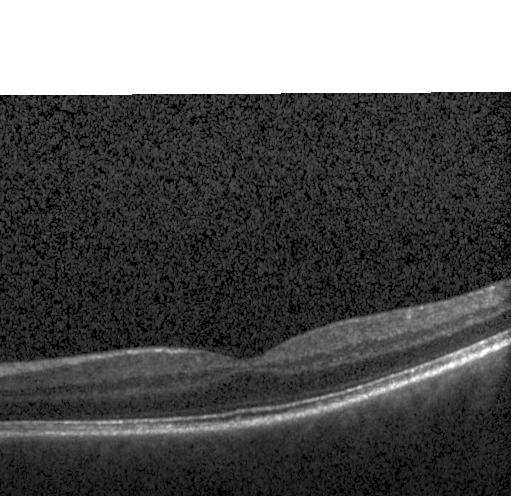

Retinal OCT cross-section; macular scan; spectral-domain optical coherence tomography; acquired on a Heidelberg Spectralis. OCT finding: no choroidal neovascularization, diabetic macular edema, or drusen.